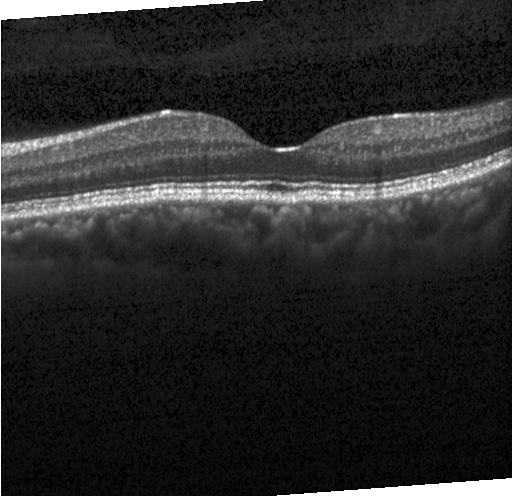

Finding: no choroidal neovascularization, no diabetic macular edema, and no drusen.